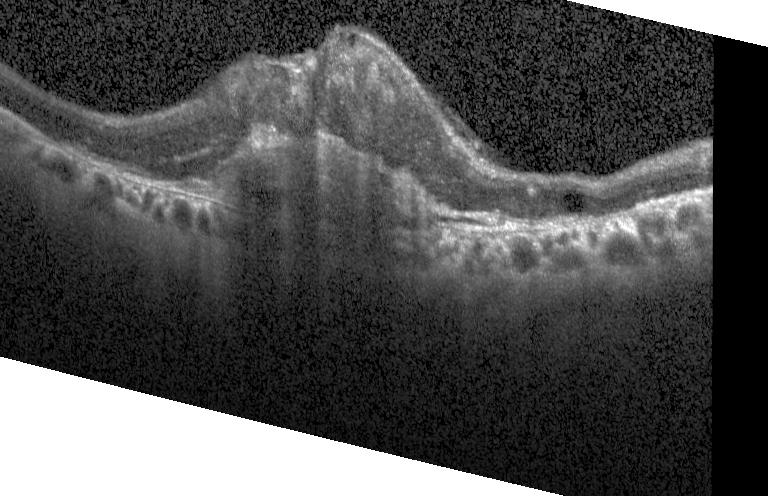 Macular scan · retinal OCT cross-section · instrument: Heidelberg Spectralis.
Assessment: a choroidal neovascular membrane.